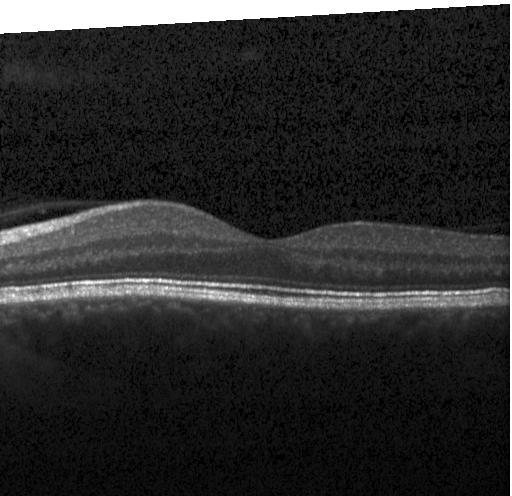
Optical coherence tomography scan · Heidelberg Spectralis. Assessment: neither choroidal neovascularization, diabetic macular edema, nor drusen.